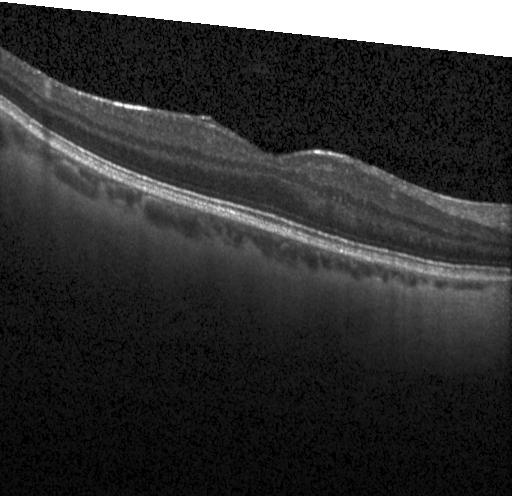 Optical coherence tomography B-scan; acquired on a Heidelberg Spectralis; spectral-domain OCT; horizontal scan through the fovea
Assessment: no evidence of choroidal neovascularization, diabetic macular edema, or drusen.